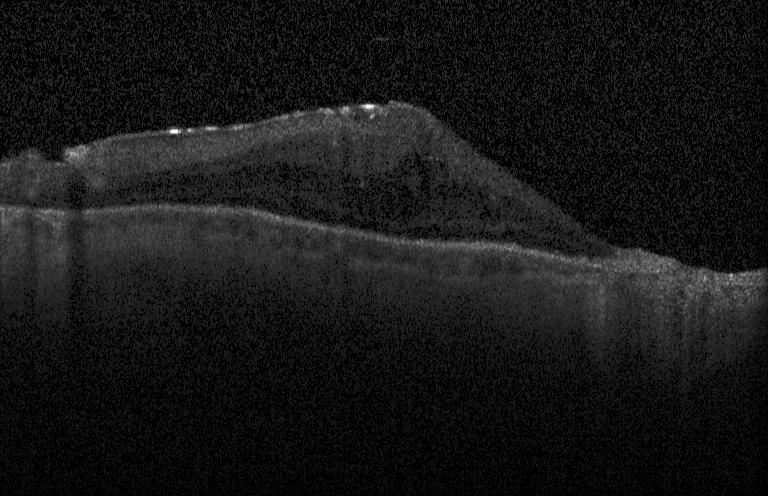

Dx: CNV.